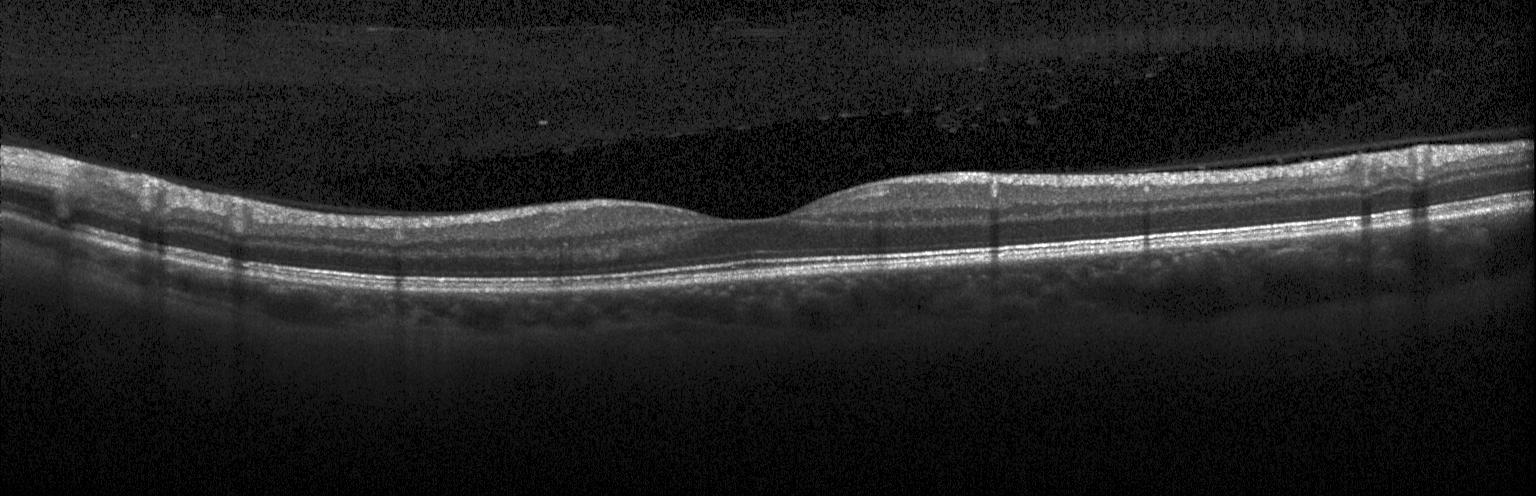
Heidelberg Spectralis · centered on the fovea · optical coherence tomography B-scan.
This B-scan demonstrates no CNV, DME, or drusen.